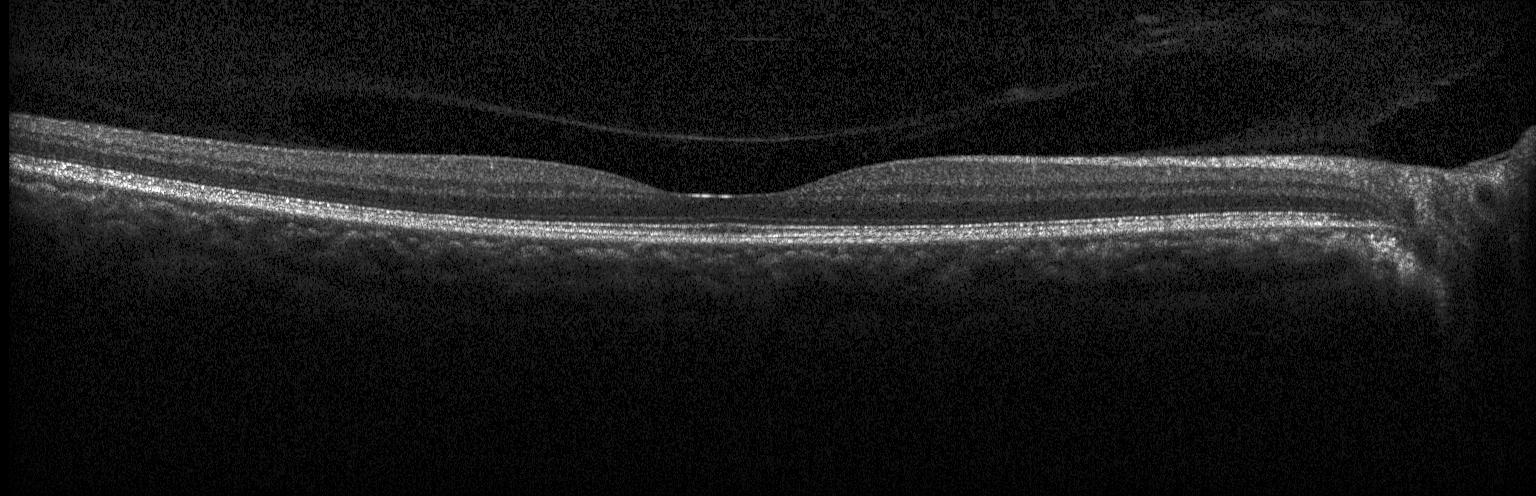 OCT B-scan.
No evidence of CNV, DME, or drusen.